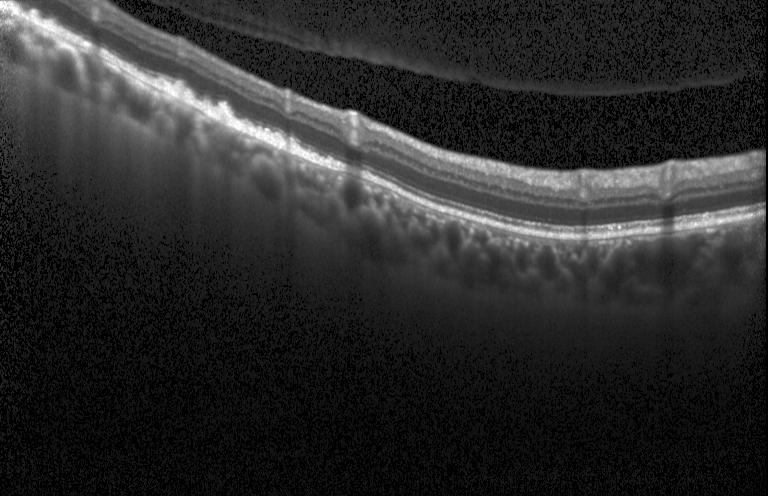 Heidelberg Spectralis OCT system; optical coherence tomography B-scan; horizontal scan through the fovea; spectral-domain OCT.
Finding: sub-RPE drusenoid deposits.